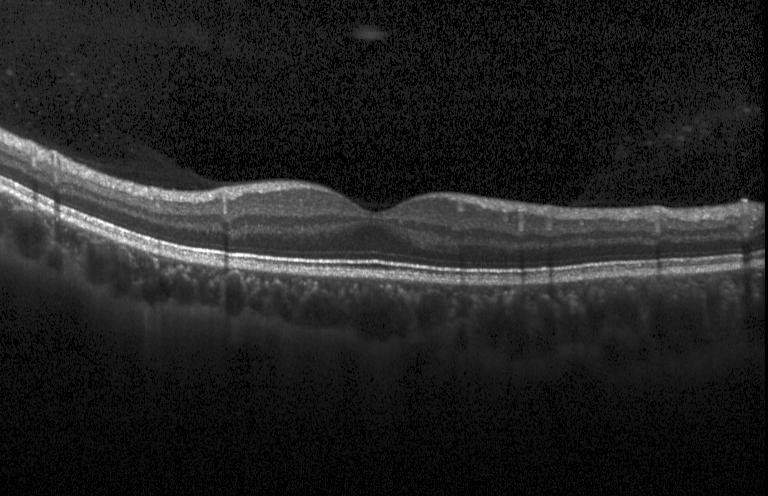
The scan shows no evidence of choroidal neovascularization, diabetic macular edema, or drusen.